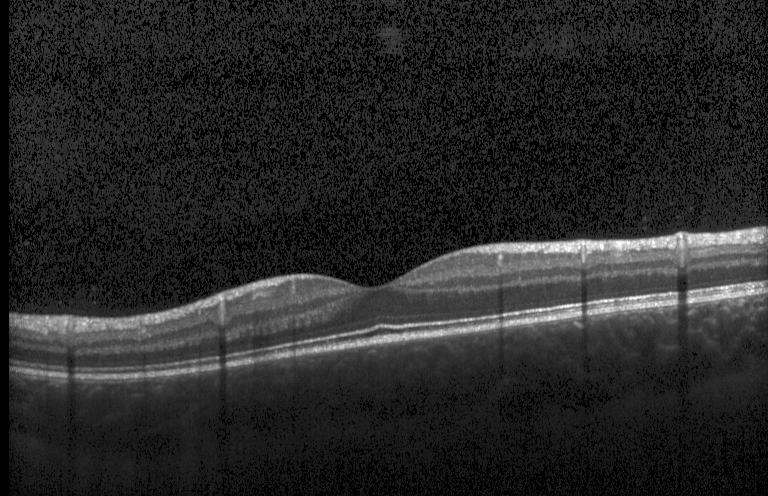

Centered on the fovea · spectral-domain optical coherence tomography · Heidelberg Spectralis OCT system · retinal OCT B-scan. The scan shows no CNV, DME, or drusen.